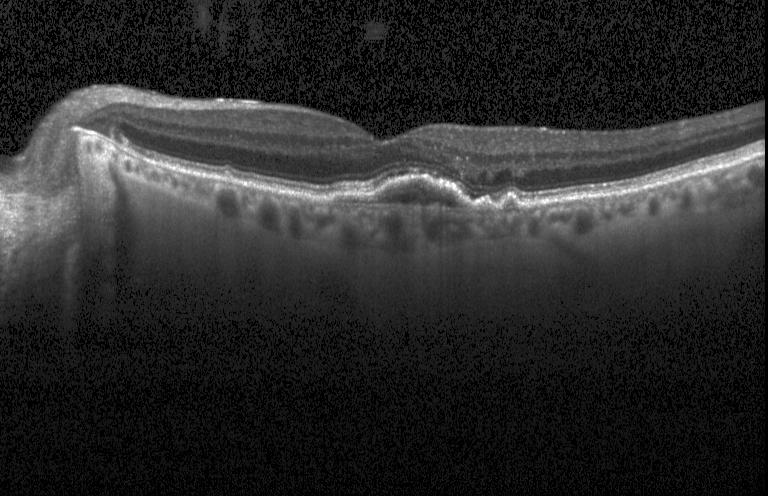 Spectral-domain OCT B-scan: a choroidal neovascular membrane.